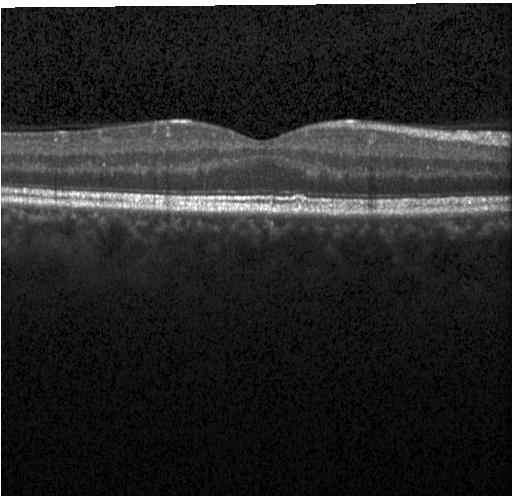 OCT B-scan — Impression: neither CNV, DME, nor drusen.